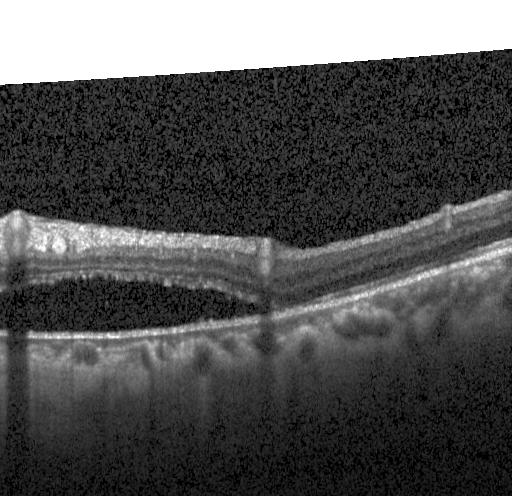
OCT finding: a choroidal neovascular membrane.